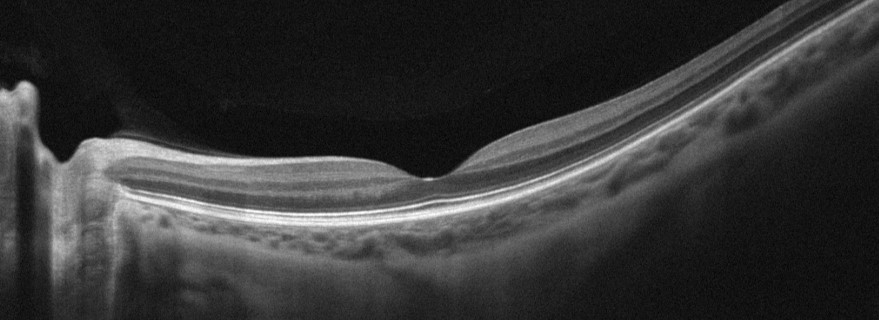
Fovea-centered · instrument: Optovue Avanti RTVue XR · retinal OCT cross-section. Assessment: no evidence of AMD, DME, ERM, RAO, RVO, or VID.